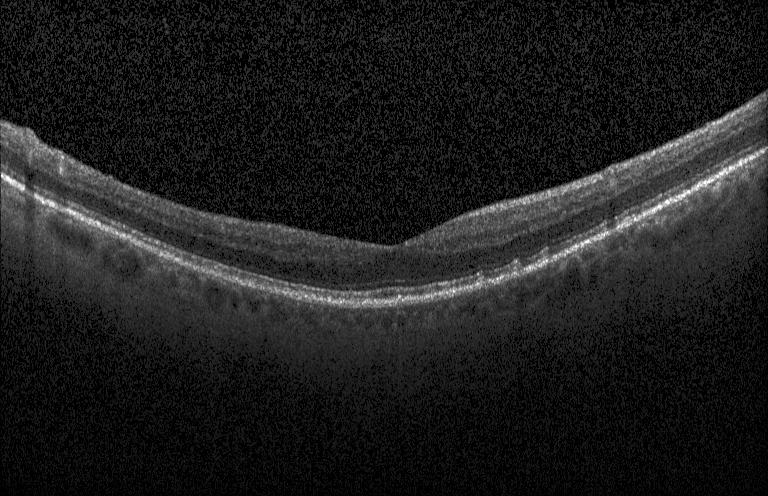

Spectral-domain OCT · OCT B-scan
OCT finding: multiple drusen.